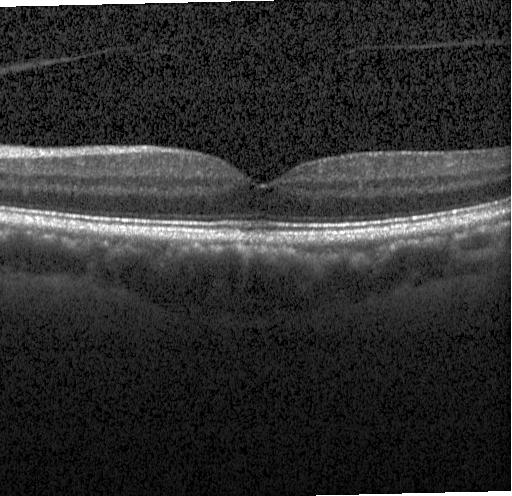
Optical coherence tomography scan · spectral-domain OCT · macular scan · Heidelberg Spectralis
Finding: no choroidal neovascularization, diabetic macular edema, or drusen.